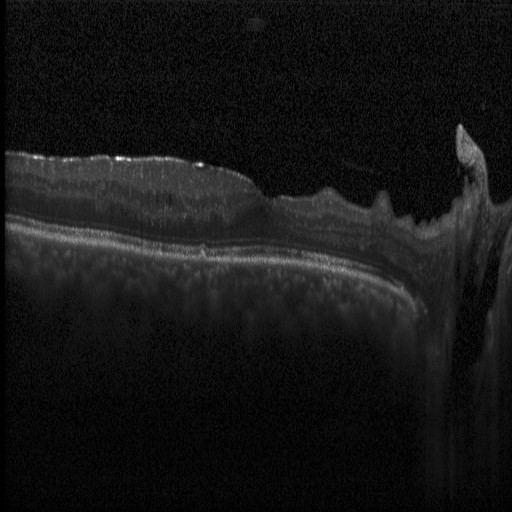 Optical coherence tomography scan. DME.